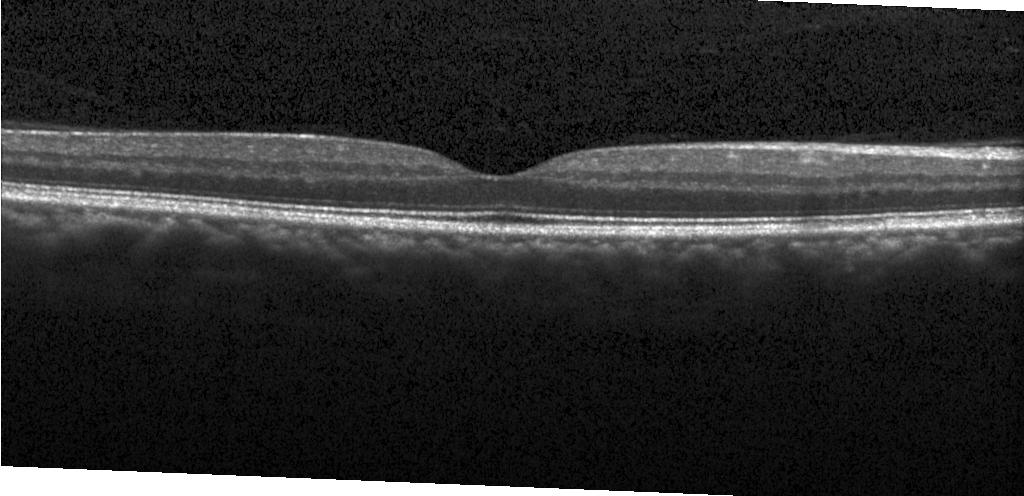

OCT scan showing no evidence of choroidal neovascularization, diabetic macular edema, or drusen.